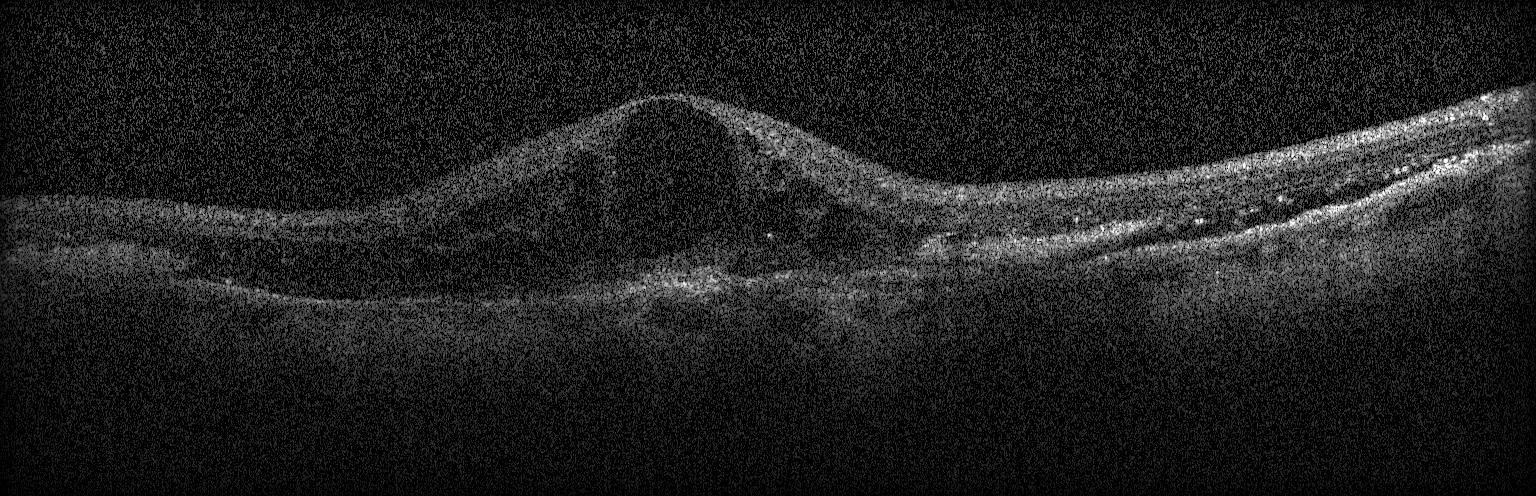
Retinal OCT cross-section · Heidelberg Spectralis.
CNV.